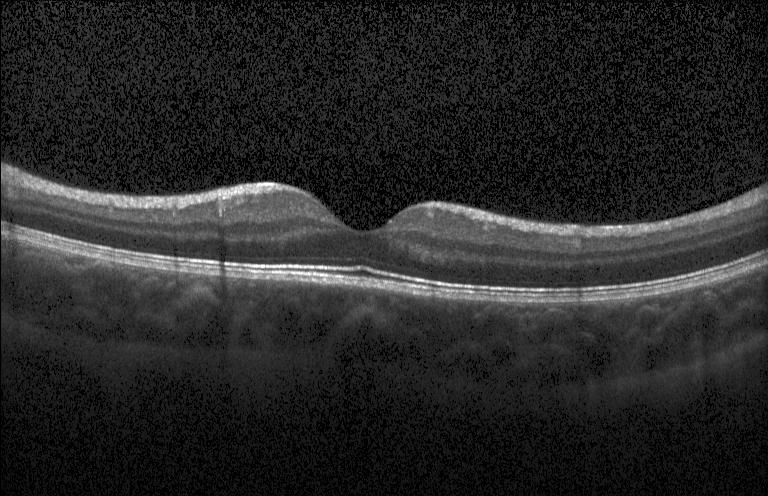
Retinal OCT cross-section — Diagnosis: no choroidal neovascularization, diabetic macular edema, or drusen.